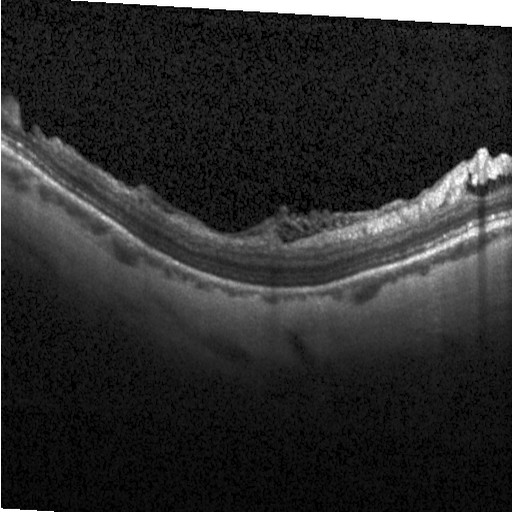 The scan shows DME.